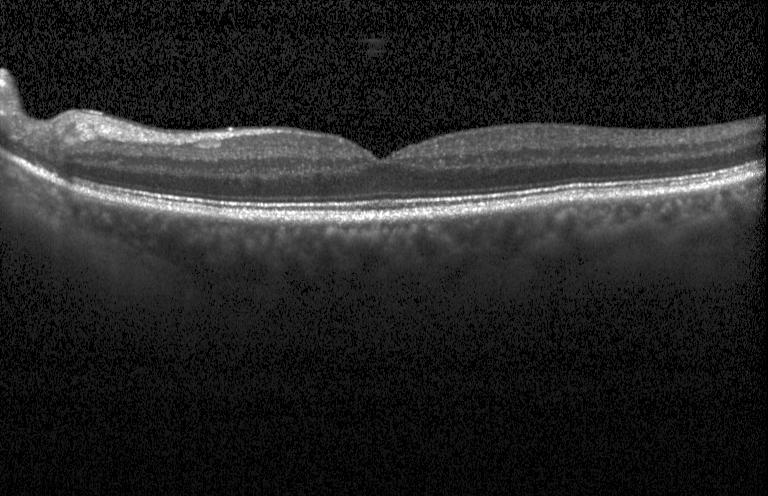 Retinal OCT B-scan. Acquired on a Heidelberg Spectralis. Through the macula. SD-OCT.
No choroidal neovascularization, diabetic macular edema, or drusen.